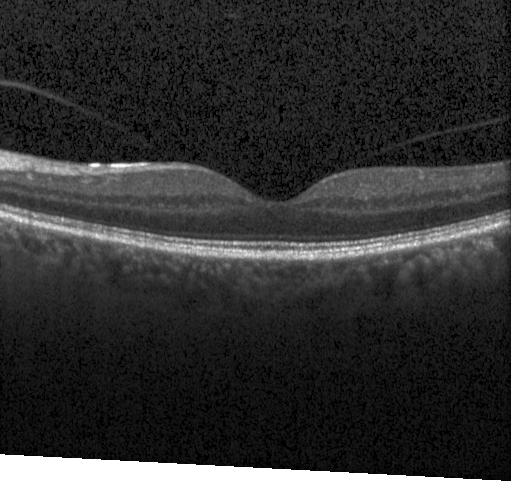

The scan shows no evidence of choroidal neovascularization, diabetic macular edema, or drusen.